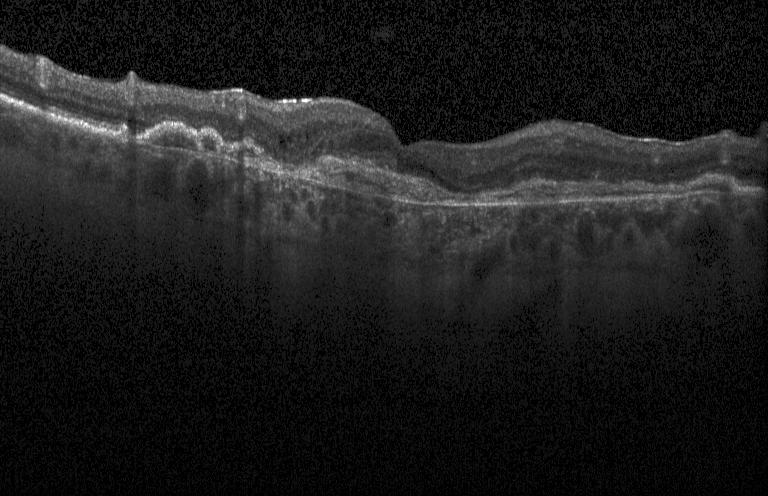
Macular scan; Heidelberg Spectralis; OCT B-scan; SD-OCT.
A choroidal neovascular membrane.